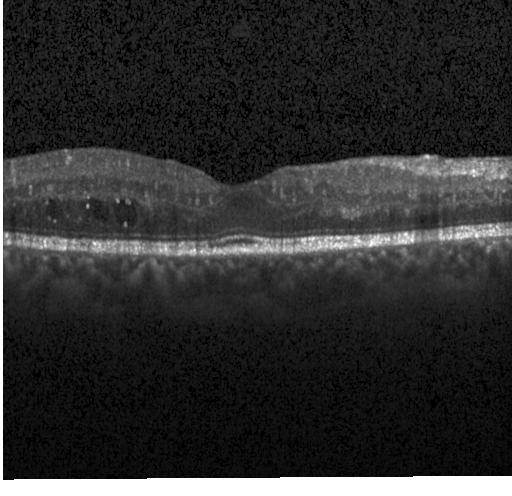

This B-scan demonstrates diabetic macular edema.